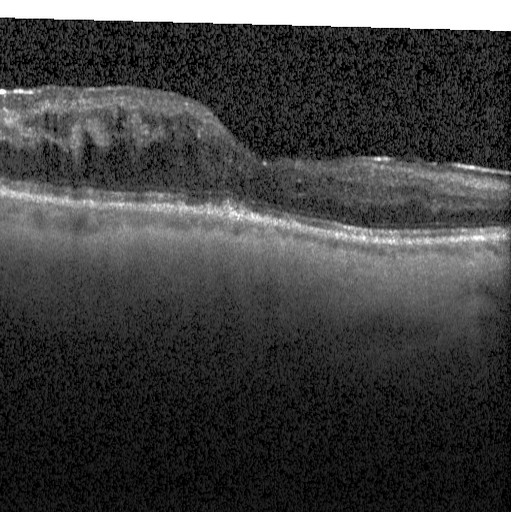 Assessment: diabetic macular edema (DME).